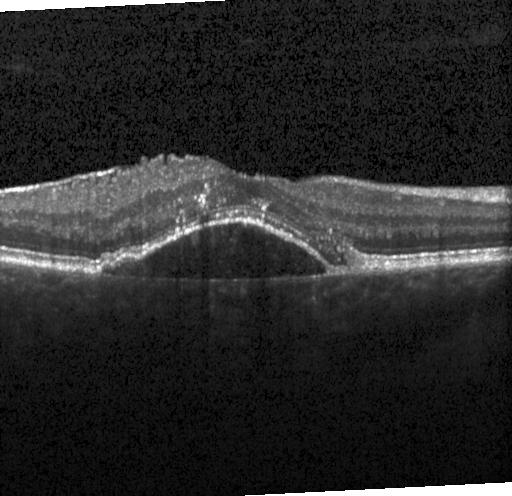

Fovea-centered; spectral-domain OCT; OCT line scan — A choroidal neovascular membrane.